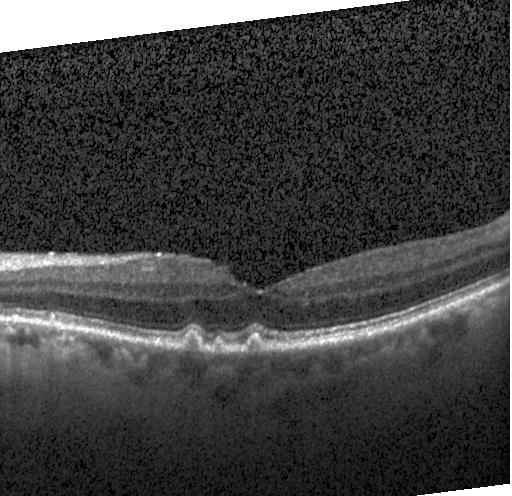 SD-OCT · instrument: Heidelberg Spectralis · OCT B-scan
Assessment: sub-RPE drusenoid deposits.